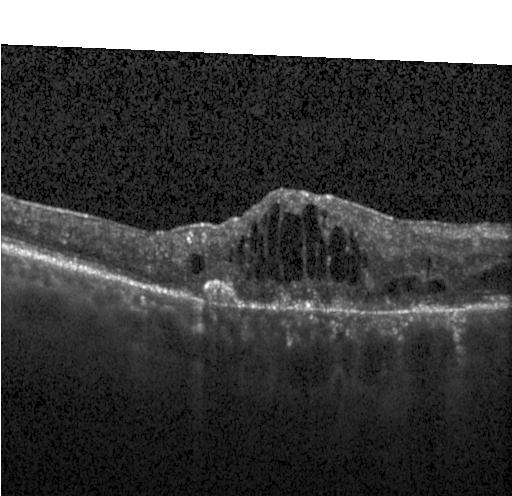 OCT line scan. Choroidal neovascularization (CNV).